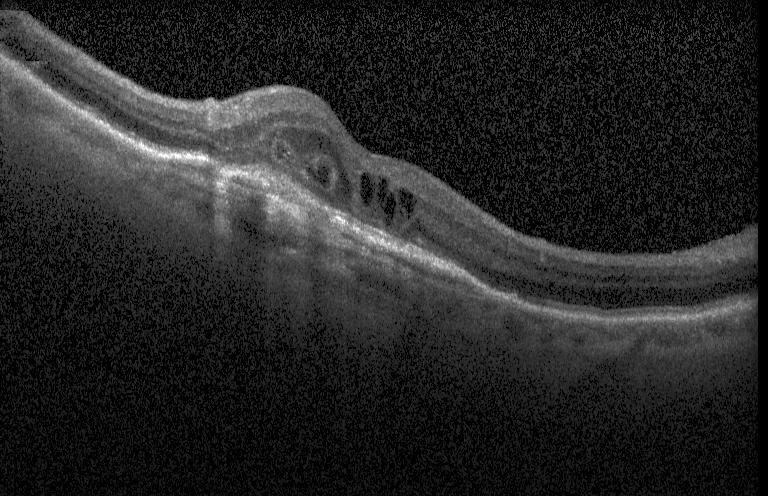

Dx: choroidal neovascularization.